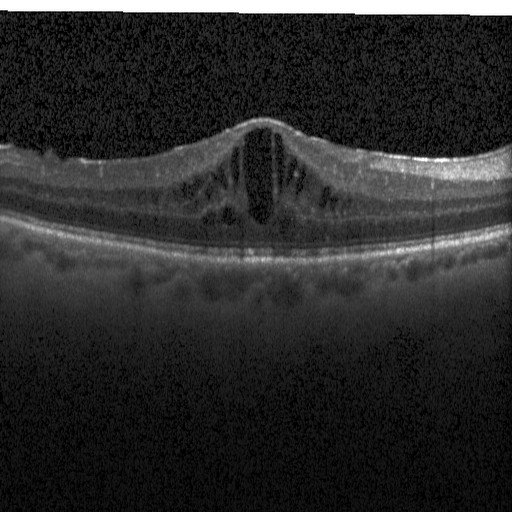 Through the macula. Heidelberg Spectralis. Optical coherence tomography B-scan
Assessment: diabetic macular edema (DME).